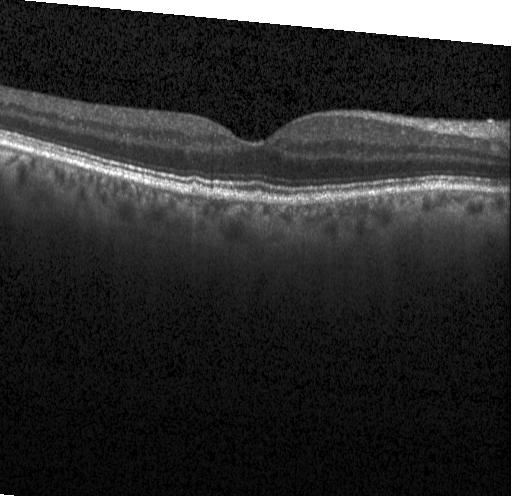
Instrument: Heidelberg Spectralis; spectral-domain OCT; optical coherence tomography B-scan; fovea-centered
Dx: sub-RPE drusenoid deposits.